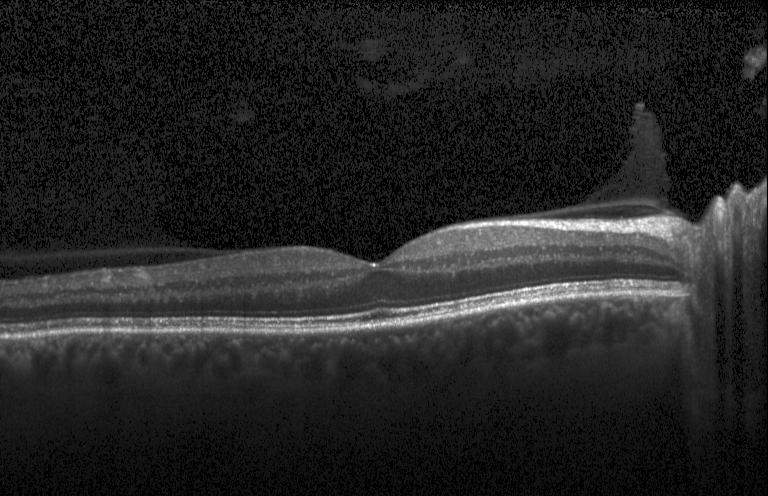
Diagnosis: neither choroidal neovascularization, diabetic macular edema, nor drusen.